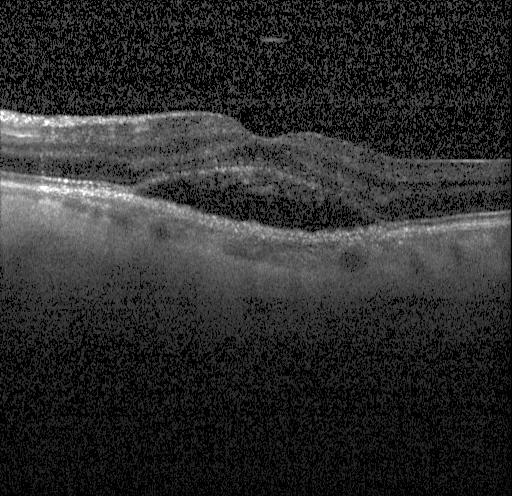 OCT line scan; centered on the fovea — Finding: a choroidal neovascular membrane.